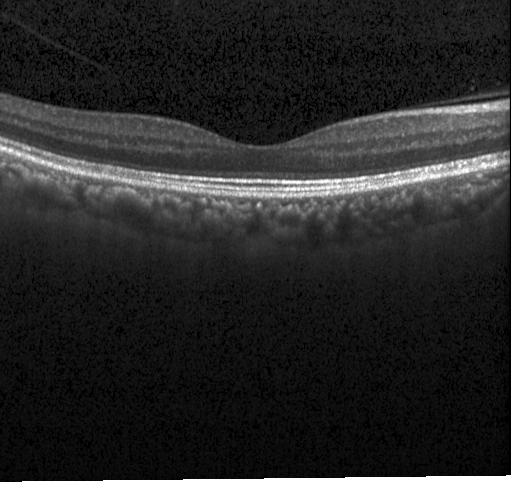

Optical coherence tomography scan. Impression: no choroidal neovascularization, diabetic macular edema, or drusen.